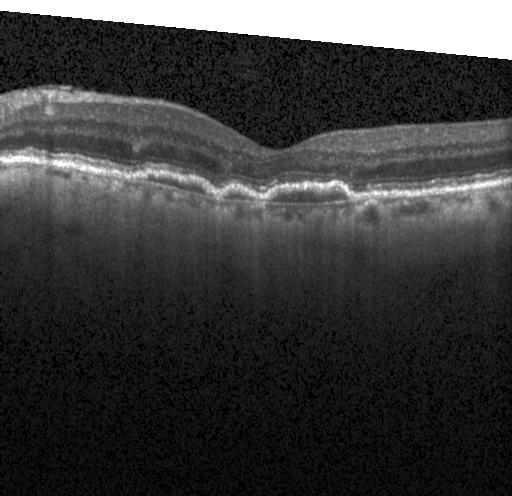 Heidelberg Spectralis; OCT line scan; spectral-domain OCT — A choroidal neovascular membrane.